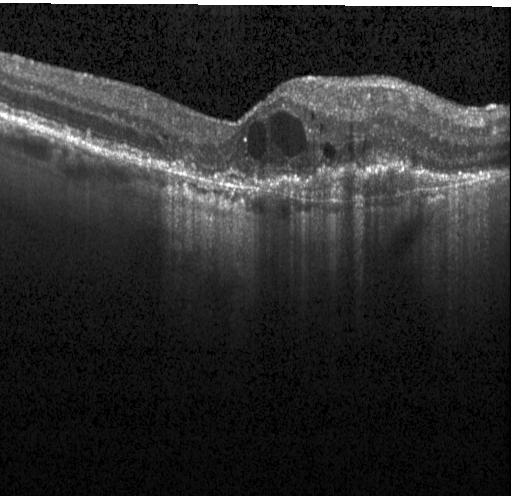

Impression: CNV.